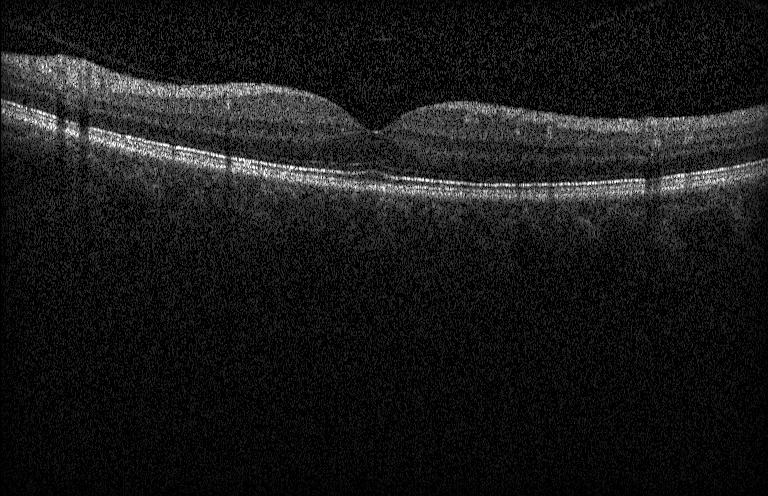 No choroidal neovascularization, no diabetic macular edema, and no drusen.